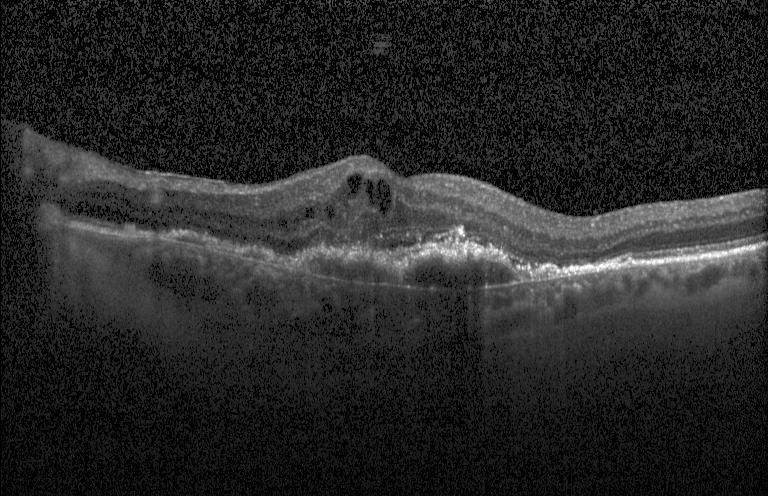 Retinal OCT cross-section, centered on the fovea. The scan shows choroidal neovascularization (CNV).